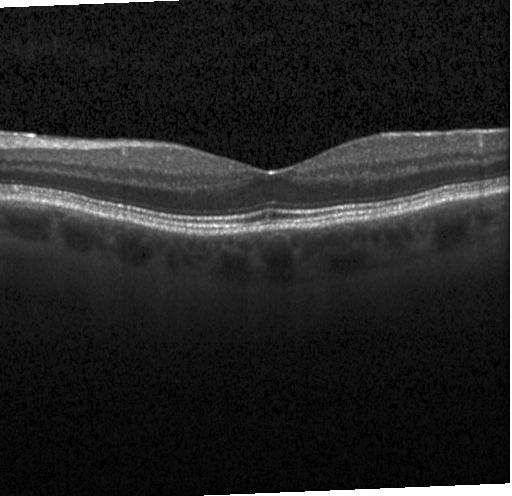
Assessment: no choroidal neovascularization, no diabetic macular edema, and no drusen.